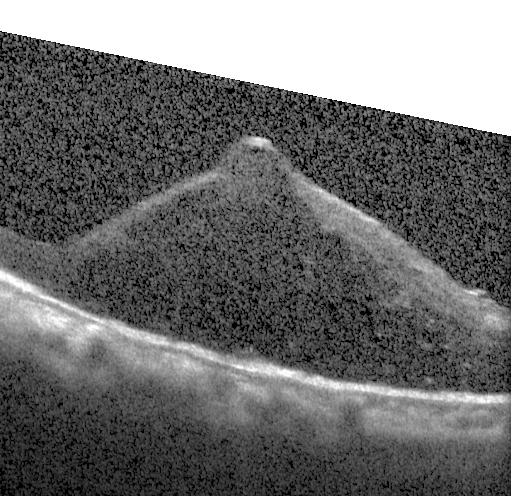 Retinal OCT cross-section showing DME.